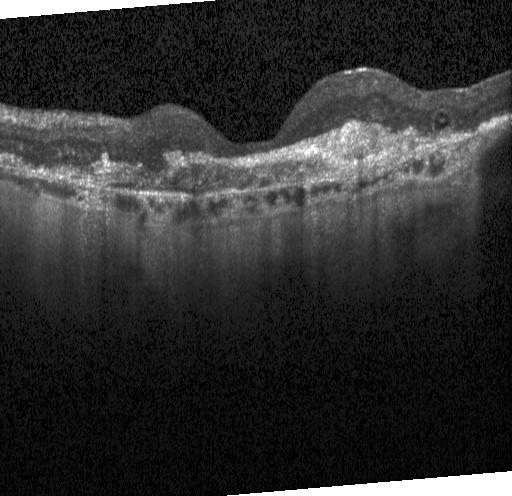 Macular OCT demonstrating CNV.